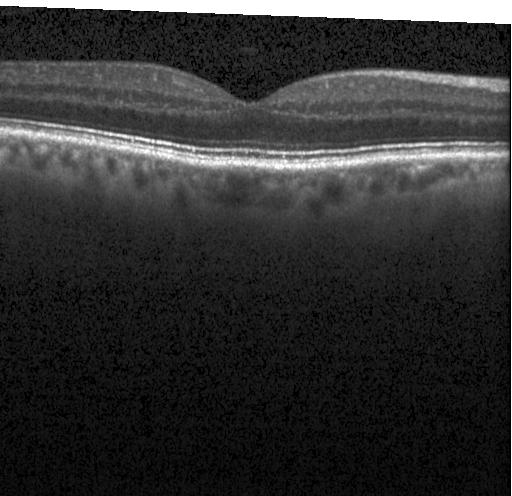
Optical coherence tomography B-scan; macular scan. Diagnosis: no evidence of CNV, DME, or drusen.